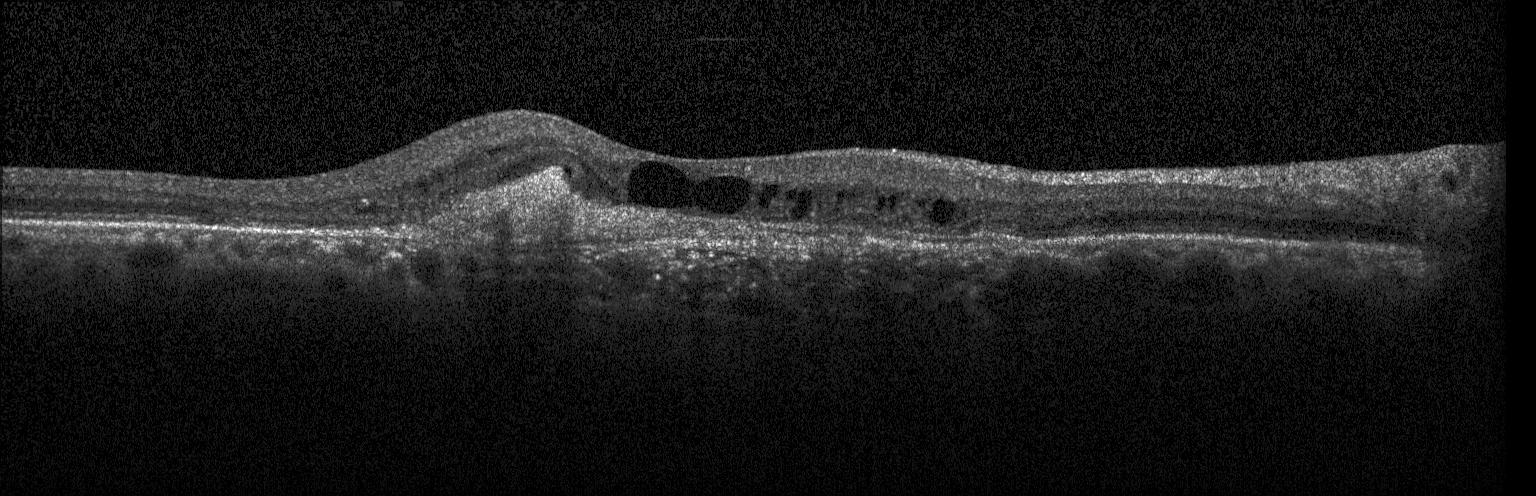

Spectral-domain optical coherence tomography, OCT B-scan, Heidelberg Spectralis OCT system, centered on the fovea. Assessment: a choroidal neovascular membrane.